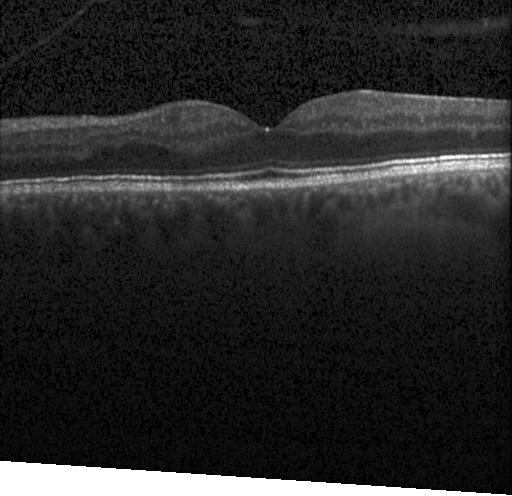 Heidelberg Spectralis OCT system. Spectral-domain optical coherence tomography. Retinal OCT B-scan. Centered on the fovea.
Assessment: no choroidal neovascularization, diabetic macular edema, or drusen.